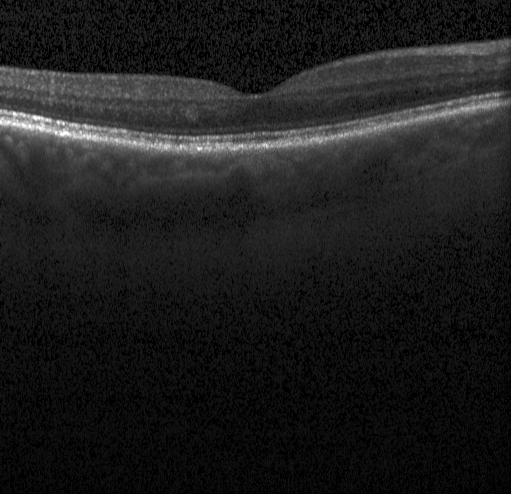 Spectral-domain OCT B-scan: no choroidal neovascularization, diabetic macular edema, or drusen.